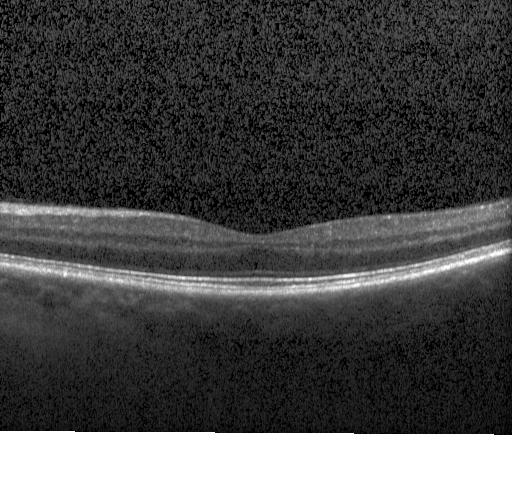

Heidelberg Spectralis, OCT B-scan
Dx: neither CNV, DME, nor drusen.